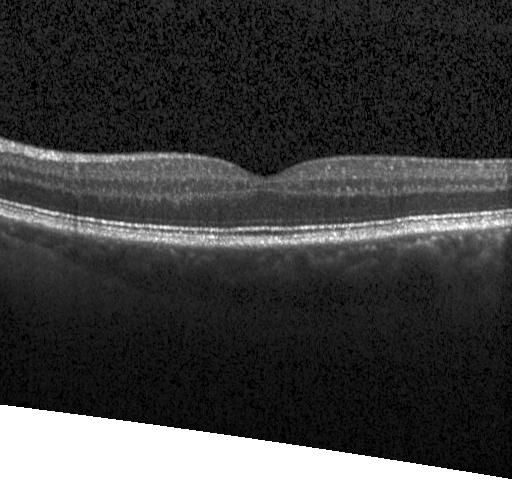

OCT finding: neither choroidal neovascularization, diabetic macular edema, nor drusen.